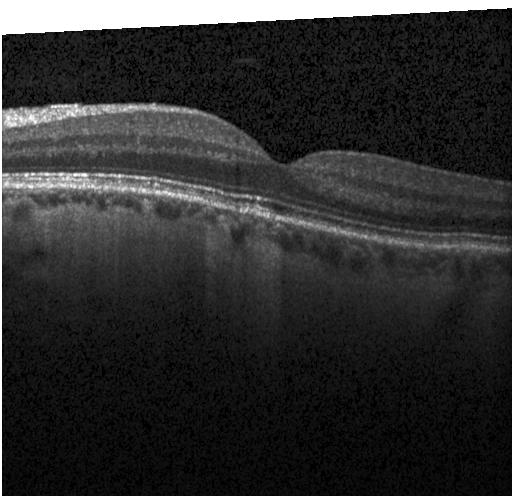

Heidelberg Spectralis · OCT B-scan · spectral-domain optical coherence tomography.
Diagnosis: no choroidal neovascularization, no diabetic macular edema, and no drusen.